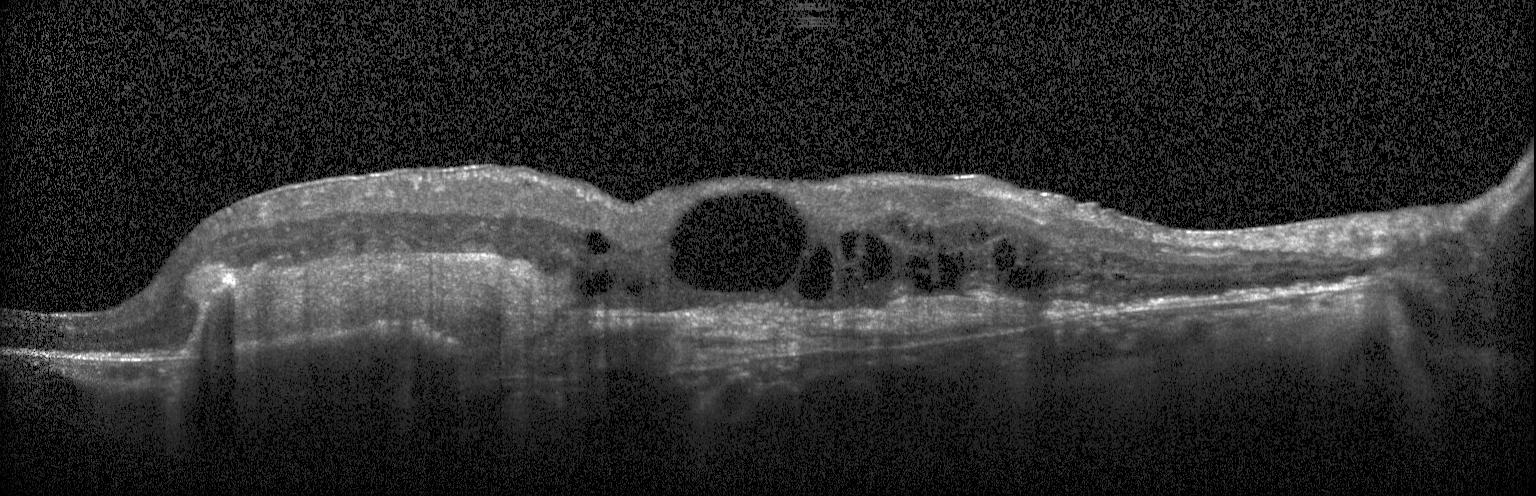 A choroidal neovascular membrane.